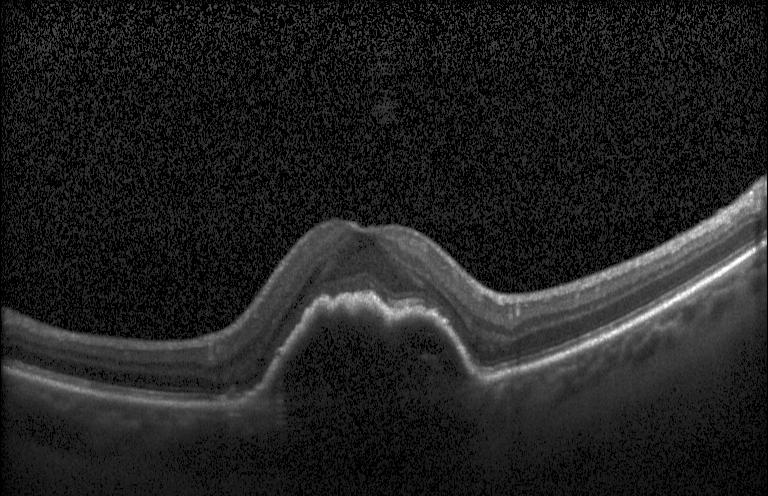

OCT line scan.
The scan shows choroidal neovascularization.